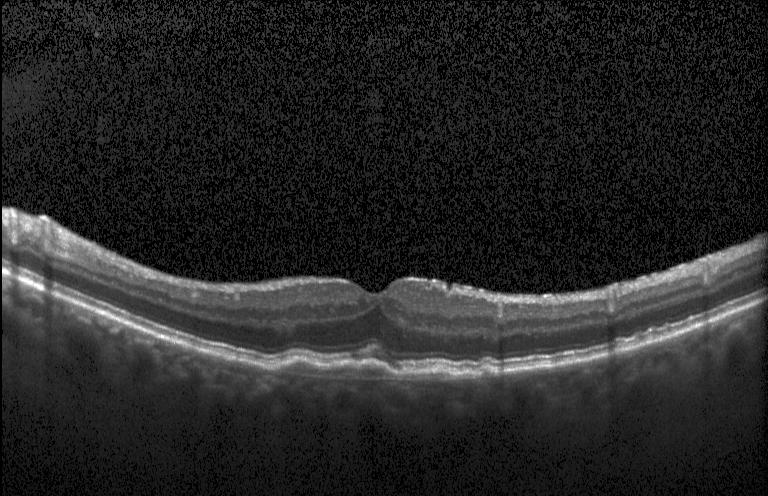 Finding: choroidal neovascularization.